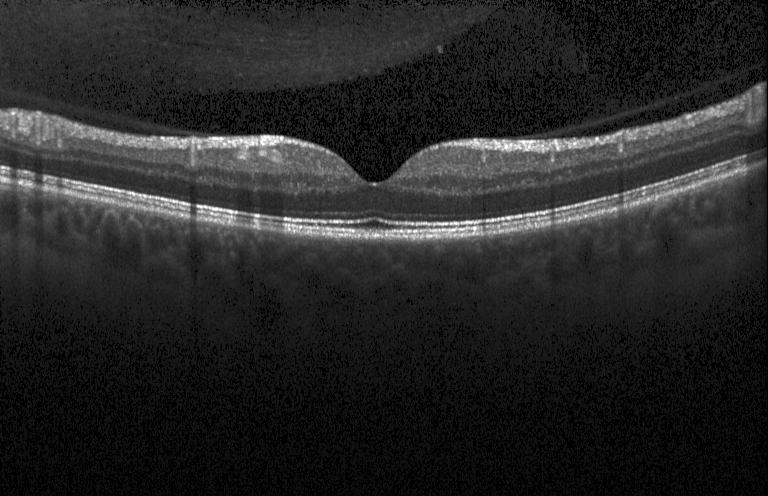

Retinal OCT cross-section showing no evidence of choroidal neovascularization, diabetic macular edema, or drusen.